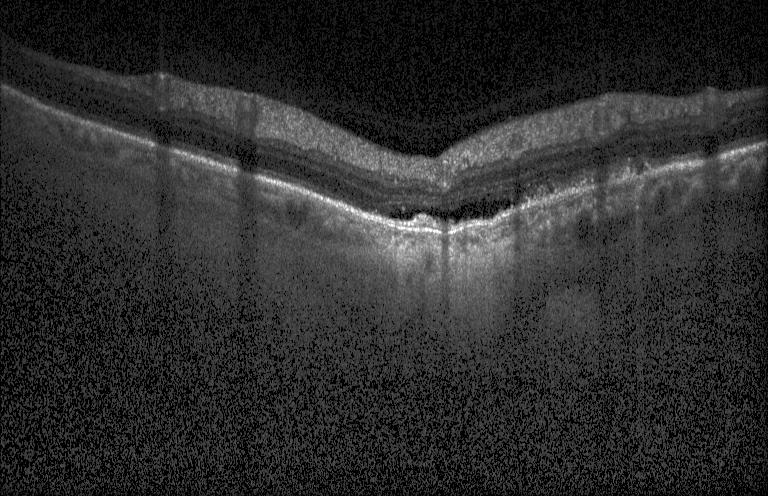 Through the macula · optical coherence tomography scan. Impression: a choroidal neovascular membrane.